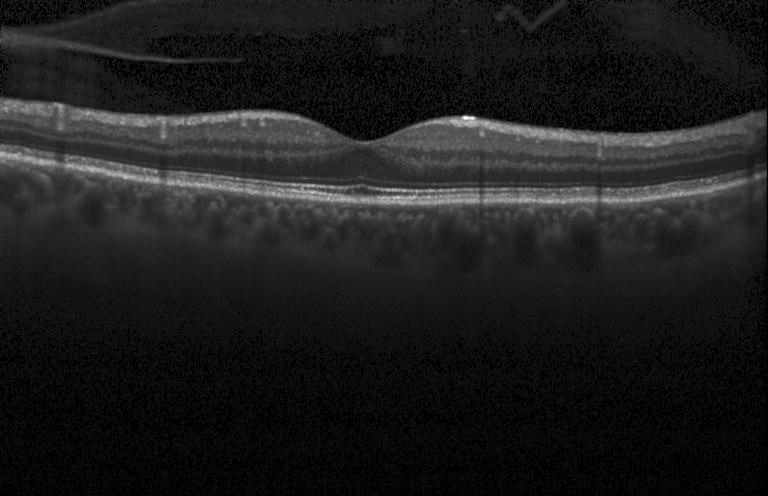
Through the macula, spectral-domain OCT, OCT line scan, Heidelberg Spectralis OCT system. Assessment: no choroidal neovascularization, diabetic macular edema, or drusen.